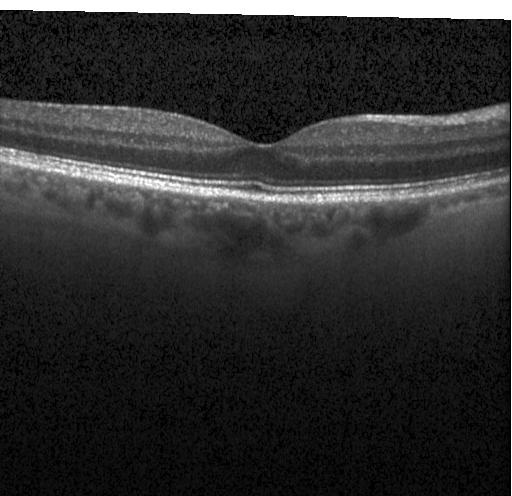

Spectral-domain OCT B-scan: no CNV, no DME, and no drusen.